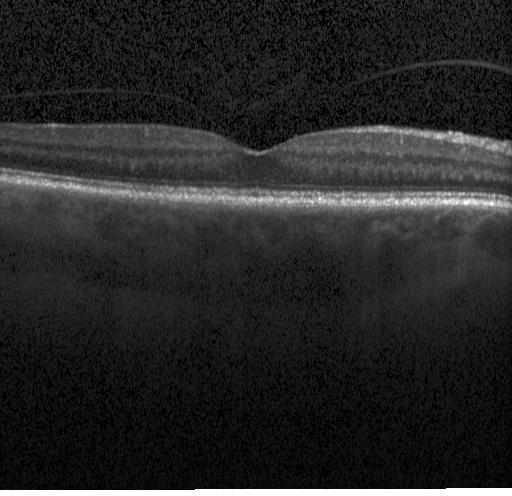 Spectral-domain OCT B-scan: no choroidal neovascularization, diabetic macular edema, or drusen.